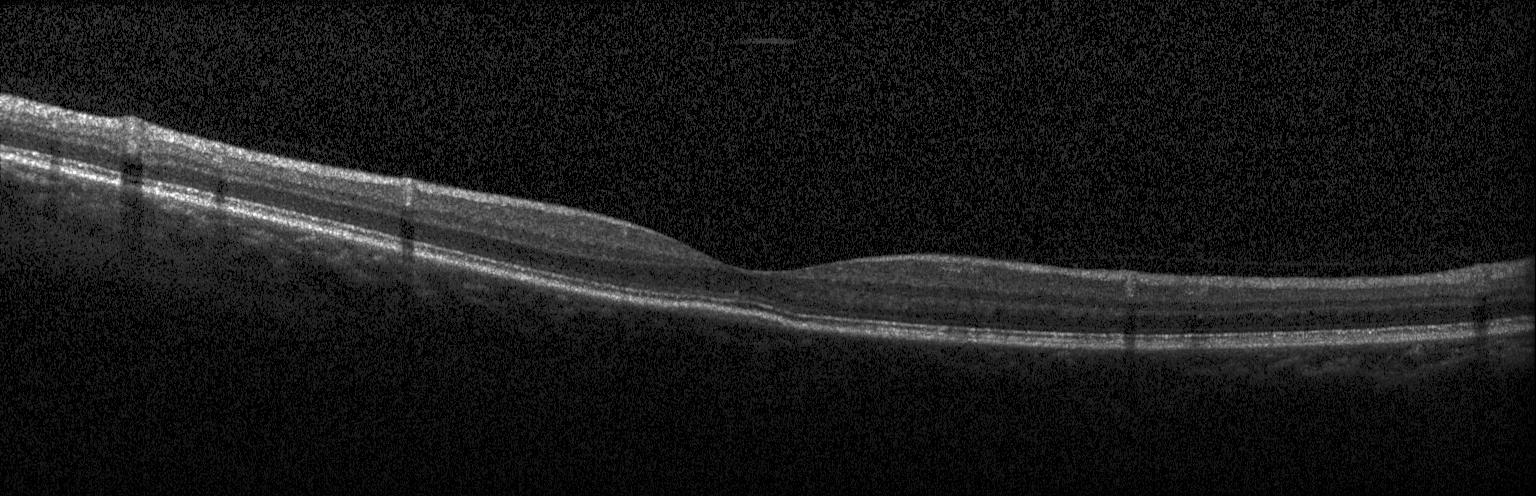 Acquired on a Heidelberg Spectralis, retinal OCT B-scan, spectral-domain OCT.
Macular OCT: no CNV, no DME, and no drusen.